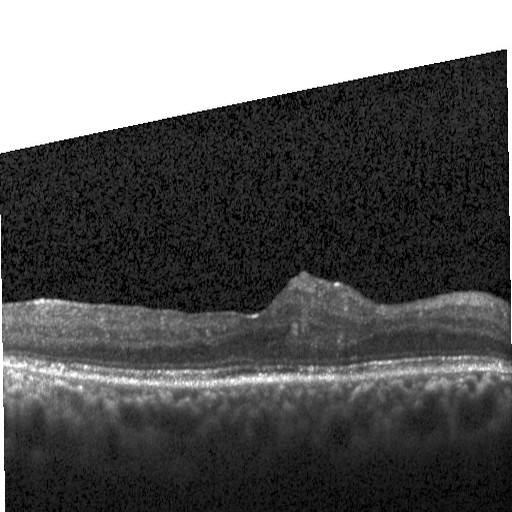
OCT line scan — OCT finding: diabetic macular edema (DME).